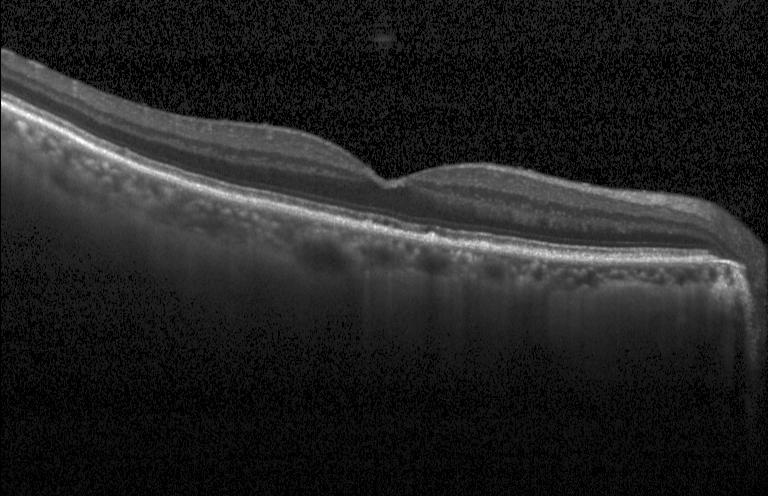
Retinal OCT cross-section showing no choroidal neovascularization, diabetic macular edema, or drusen.